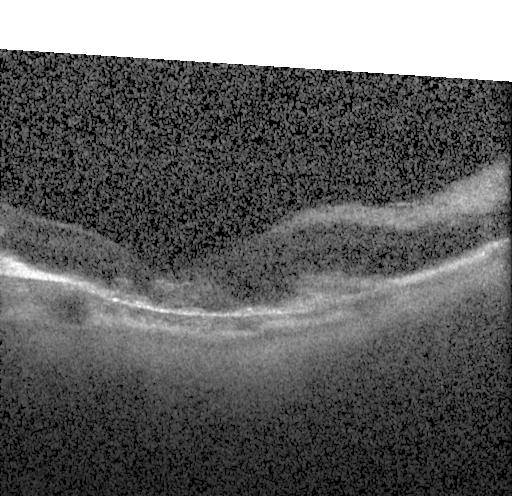

OCT finding: a choroidal neovascular membrane.